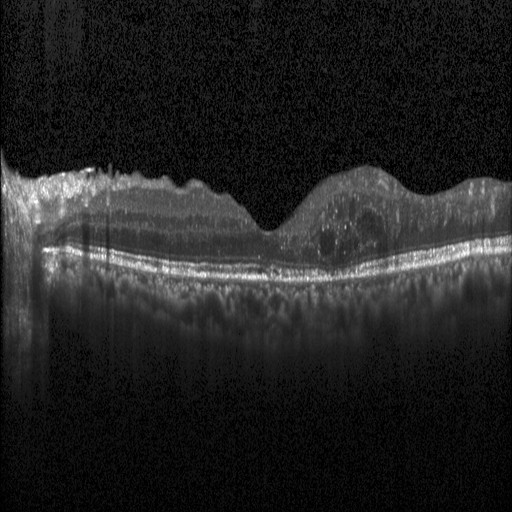 Optical coherence tomography B-scan. Macular OCT: diabetic macular edema.